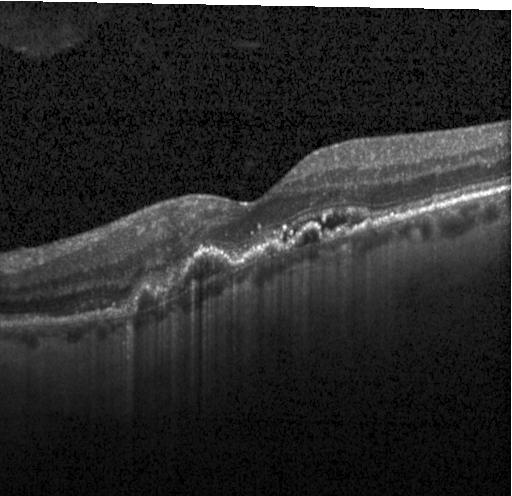 Diagnosis: choroidal neovascularization (CNV).